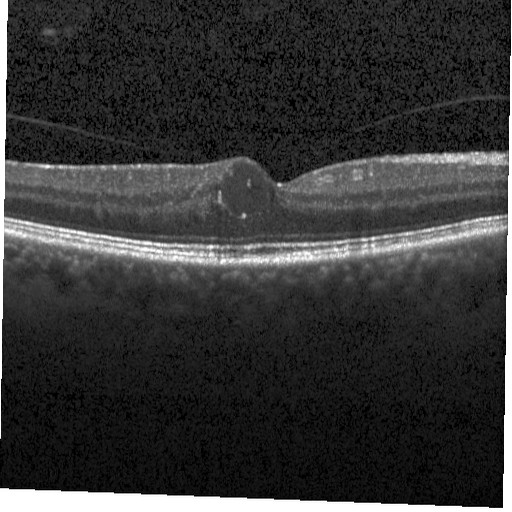 The scan shows DME.